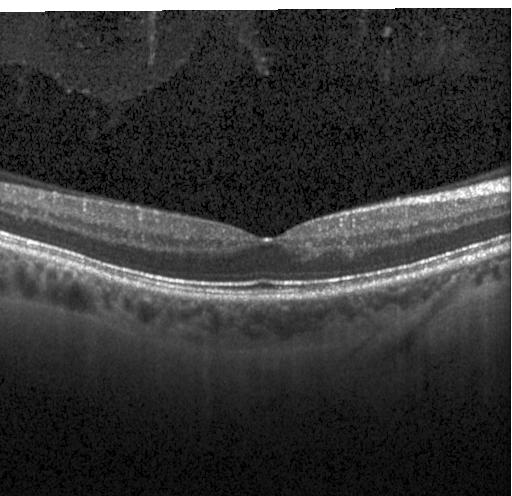

Optical coherence tomography scan. Acquired on a Heidelberg Spectralis. Spectral-domain optical coherence tomography. Centered on the fovea.
Finding: no evidence of choroidal neovascularization, diabetic macular edema, or drusen.